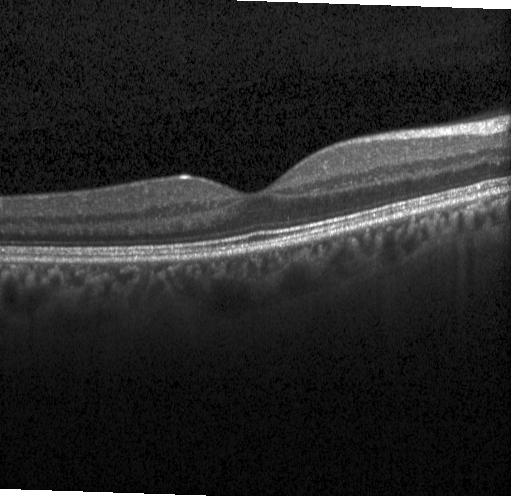

Spectral-domain OCT; Heidelberg Spectralis; macular scan; OCT line scan.
Macular OCT: no choroidal neovascularization, no diabetic macular edema, and no drusen.